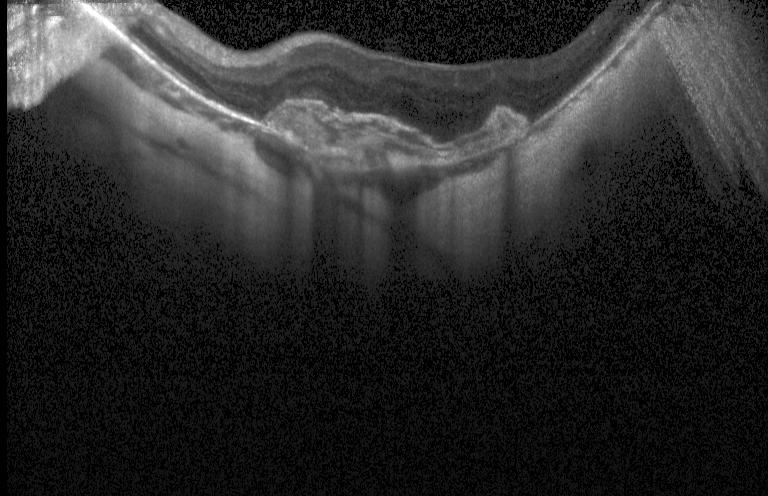
Finding: choroidal neovascularization.